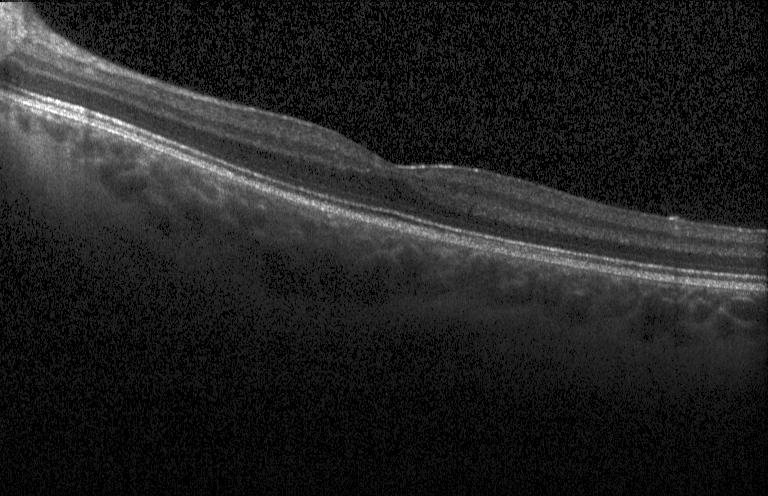 Optical coherence tomography scan · acquired on a Heidelberg Spectralis. Dx: no evidence of choroidal neovascularization, diabetic macular edema, or drusen.